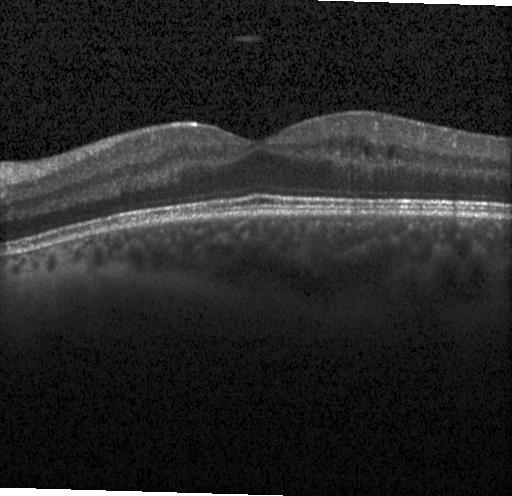

Spectral-domain OCT B-scan: diabetic macular edema (DME).